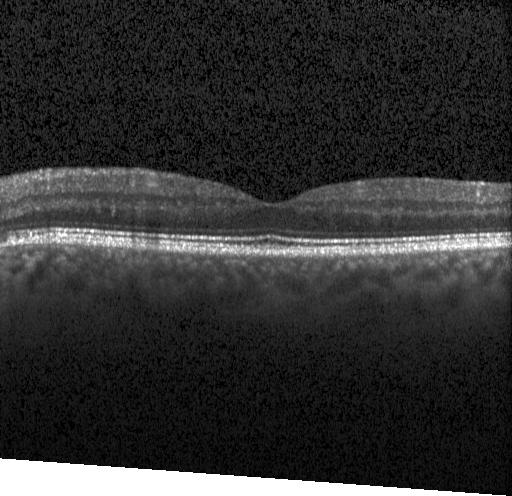
OCT B-scan; macular scan
Assessment: no evidence of CNV, DME, or drusen.